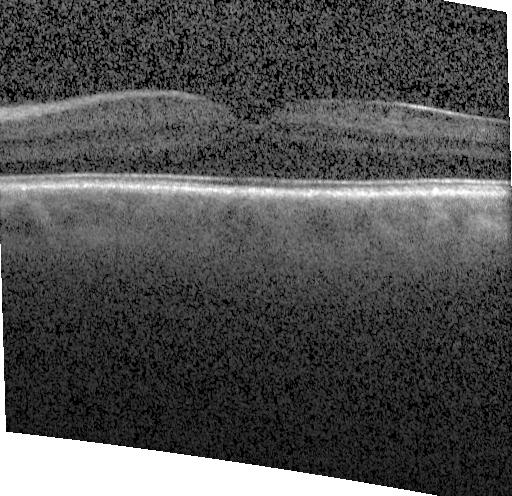 Acquired on a Heidelberg Spectralis. Retinal OCT B-scan. Spectral-domain OCT — Finding: no choroidal neovascularization, diabetic macular edema, or drusen.